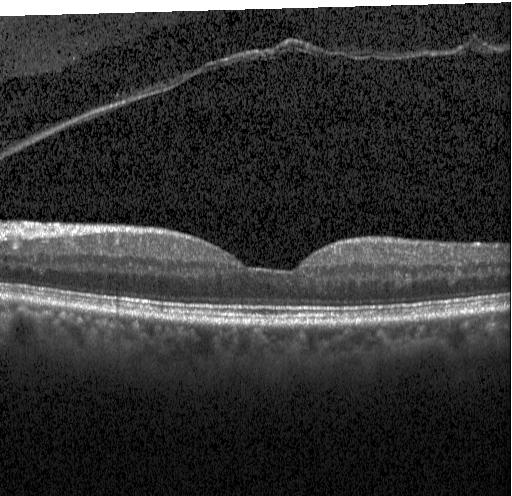

Retinal OCT B-scan; through the macula. Dx: neither choroidal neovascularization, diabetic macular edema, nor drusen.